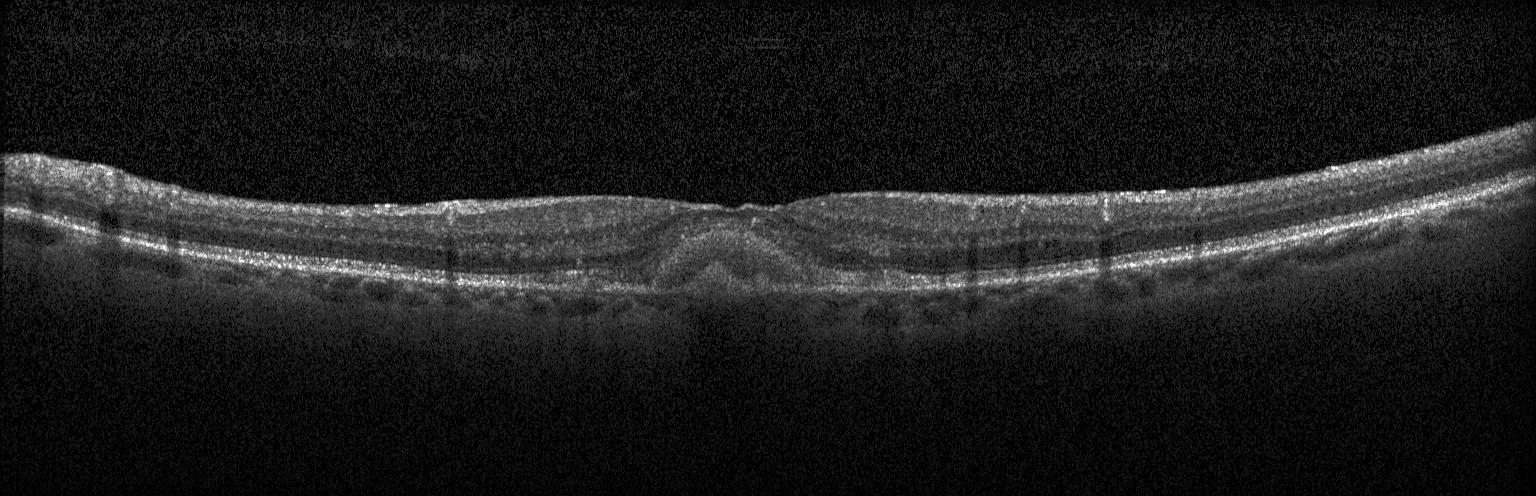
Finding: choroidal neovascularization (CNV).